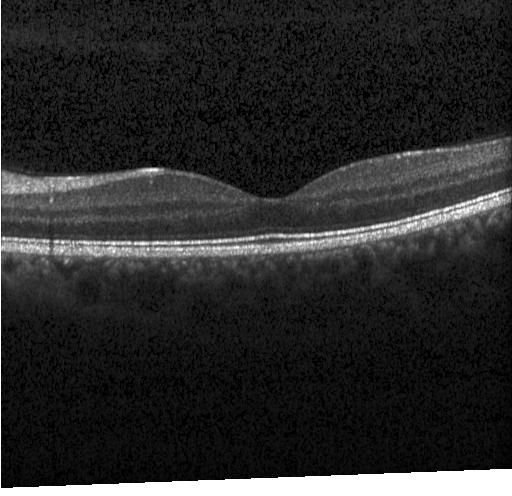 OCT finding: no CNV, no DME, and no drusen.